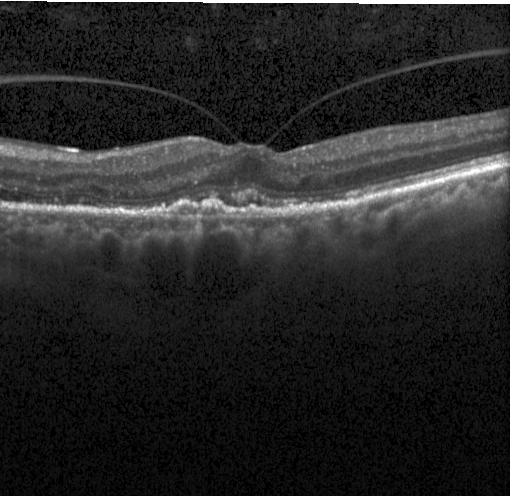
Optical coherence tomography scan · horizontal scan through the fovea — Finding: choroidal neovascularization.